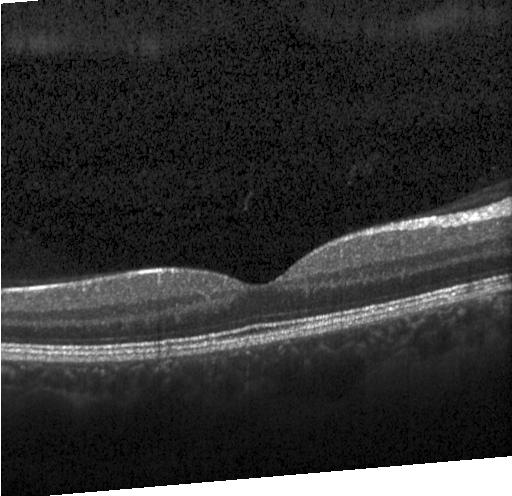
Heidelberg Spectralis, optical coherence tomography B-scan. Diagnosis: no choroidal neovascularization, no diabetic macular edema, and no drusen.